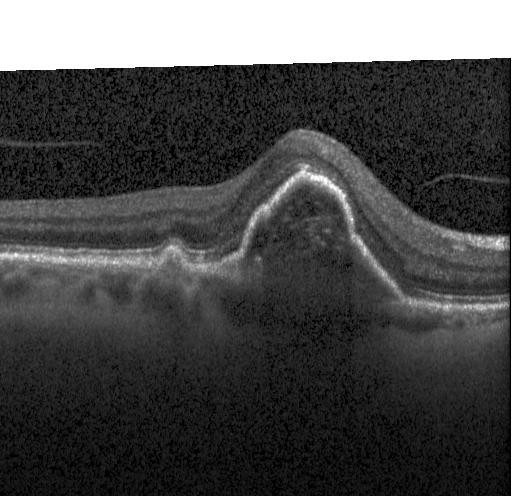
OCT finding: a choroidal neovascular membrane.